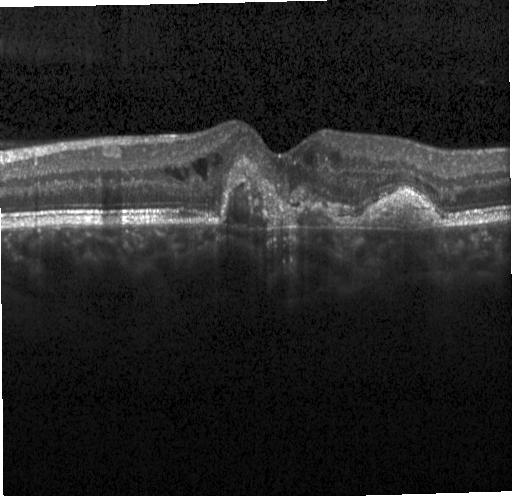
OCT B-scan · macular scan
Finding: a choroidal neovascular membrane.